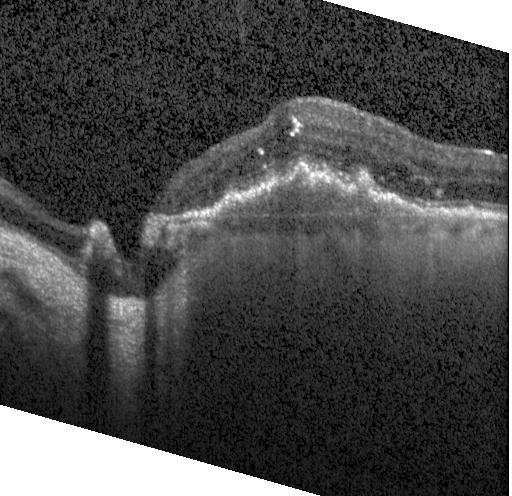

This B-scan demonstrates a choroidal neovascular membrane.